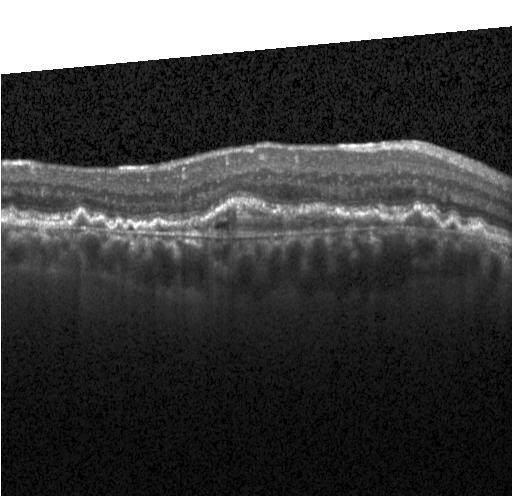
Retinal OCT B-scan
Diagnosis: choroidal neovascularization.